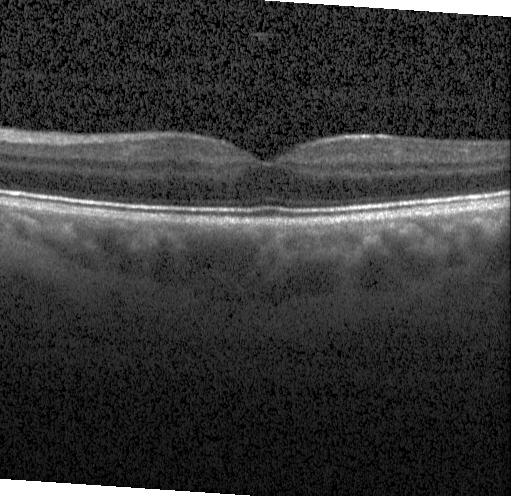 Spectral-domain OCT B-scan: no evidence of choroidal neovascularization, diabetic macular edema, or drusen.